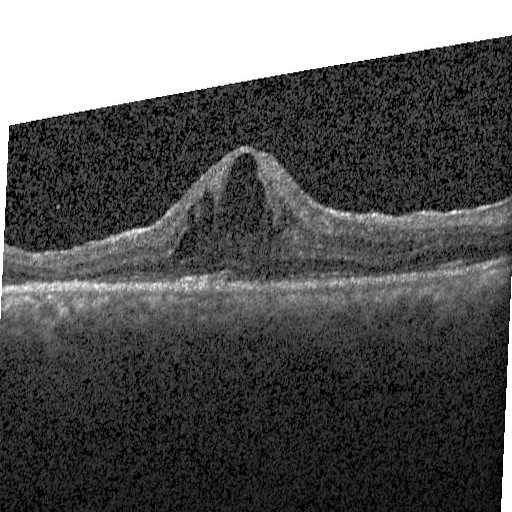
Finding: DME.